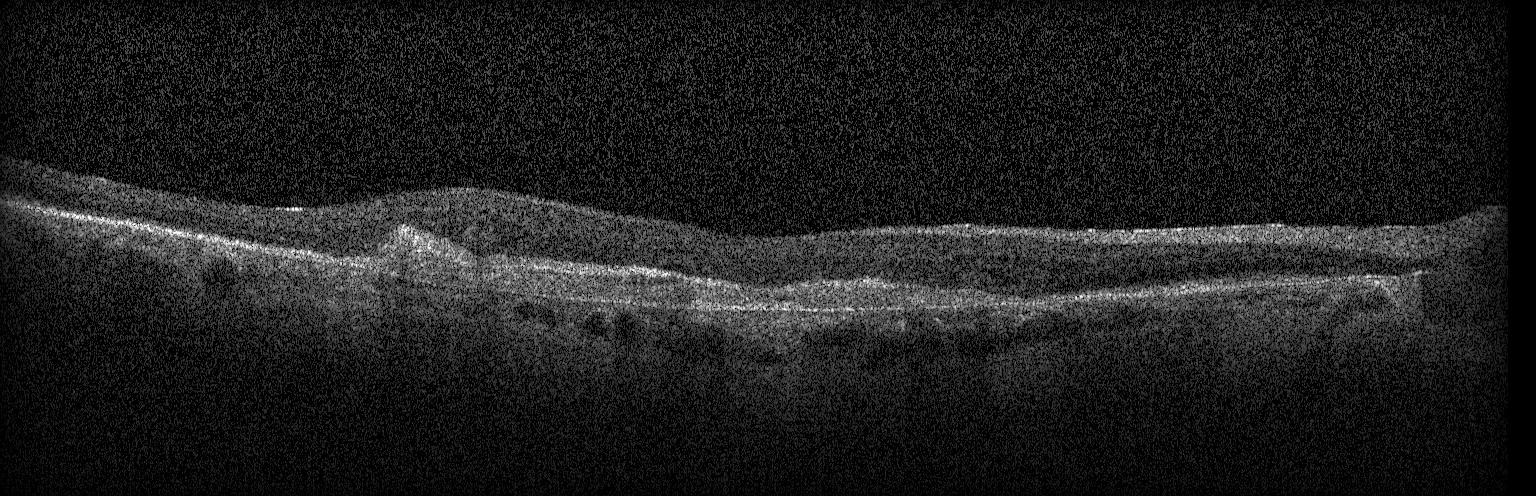 Macular scan, OCT B-scan. Finding: a choroidal neovascular membrane.